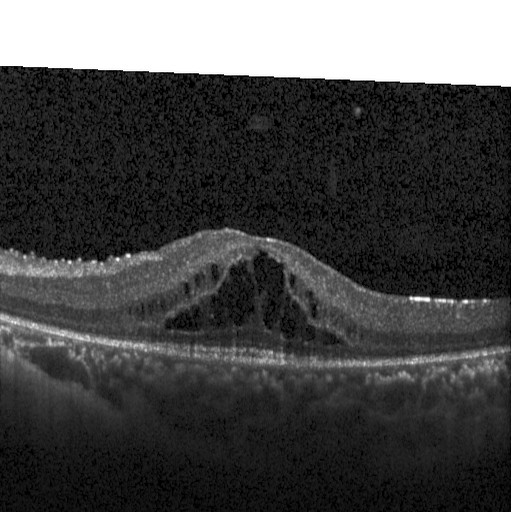

Retinal OCT cross-section
Impression: diabetic macular edema (DME).